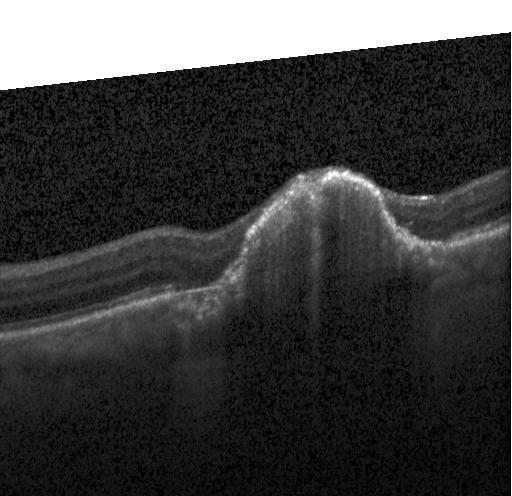
OCT B-scan. Acquired on a Heidelberg Spectralis. Through the macula — Dx: a choroidal neovascular membrane.